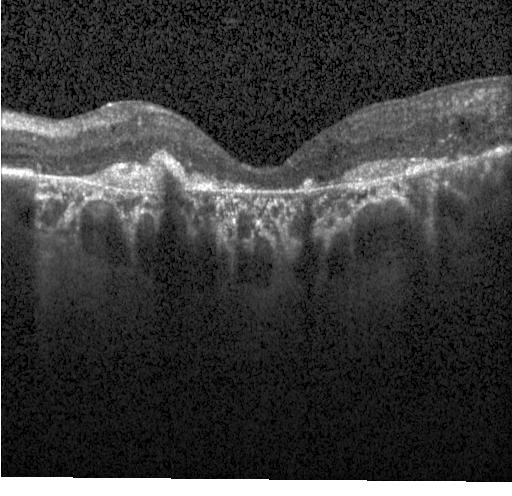
Heidelberg Spectralis OCT system, optical coherence tomography scan. Impression: CNV.